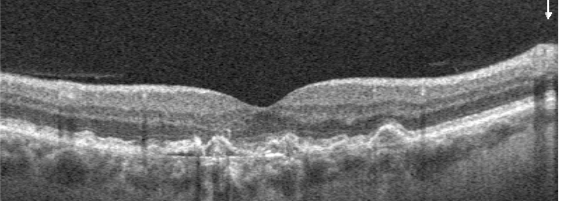 Retinal OCT cross-section.
The scan shows AMD.